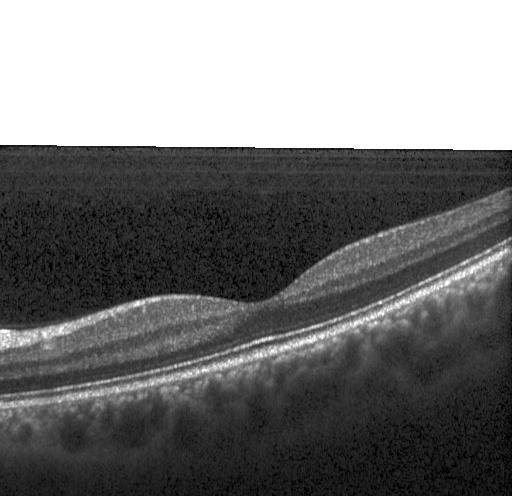 Heidelberg Spectralis; retinal OCT B-scan; spectral-domain OCT; horizontal scan through the fovea.
Impression: no evidence of choroidal neovascularization, diabetic macular edema, or drusen.